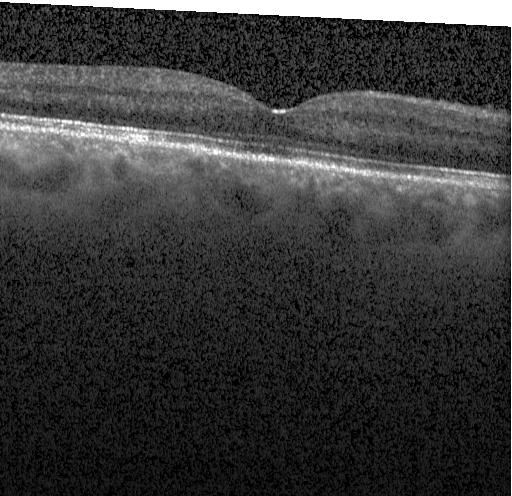
Optical coherence tomography B-scan
Diagnosis: no evidence of choroidal neovascularization, diabetic macular edema, or drusen.